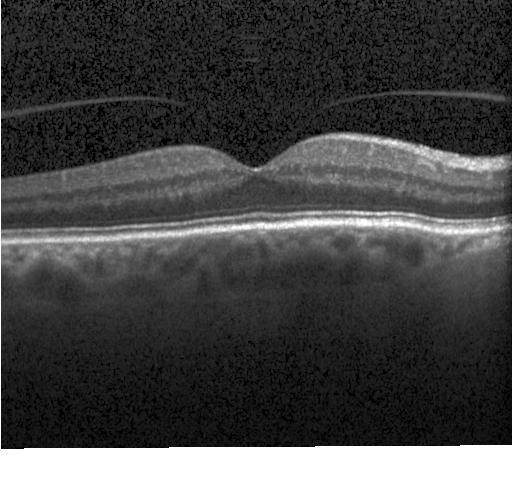
OCT line scan; Heidelberg Spectralis.
Impression: no choroidal neovascularization, no diabetic macular edema, and no drusen.